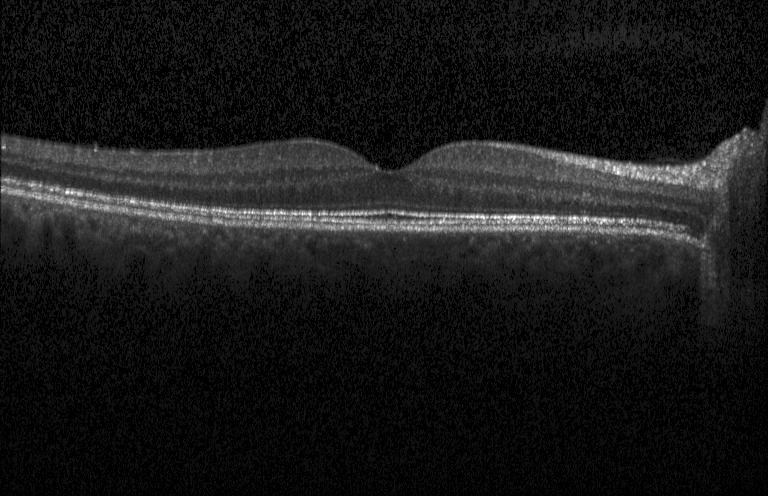
Heidelberg Spectralis OCT system · SD-OCT · fovea-centered · retinal OCT cross-section.
Macular OCT: neither choroidal neovascularization, diabetic macular edema, nor drusen.